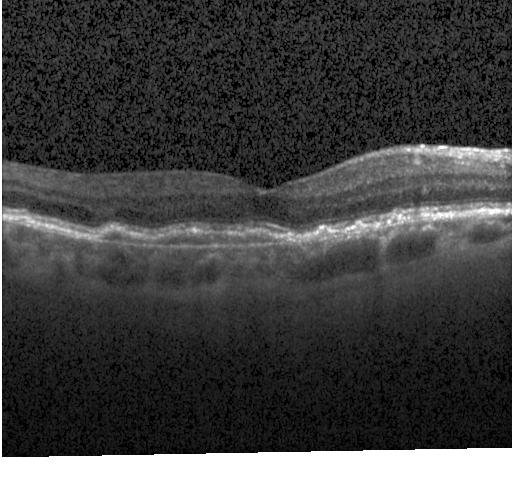
Retinal OCT B-scan.
Impression: CNV.